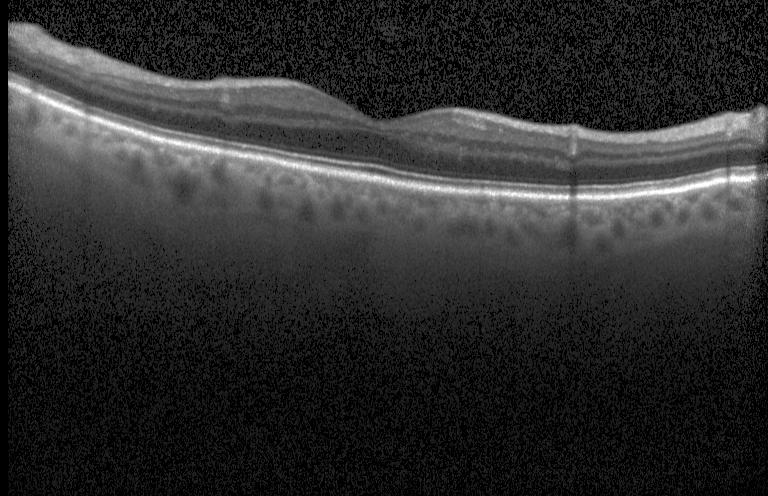

Optical coherence tomography scan. Horizontal scan through the fovea. SD-OCT. Heidelberg Spectralis.
Assessment: neither choroidal neovascularization, diabetic macular edema, nor drusen.